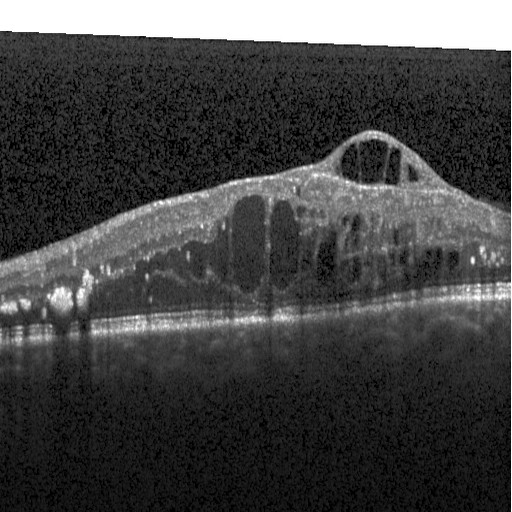 Fovea-centered, OCT line scan, acquired on a Heidelberg Spectralis, SD-OCT — Assessment: DME.